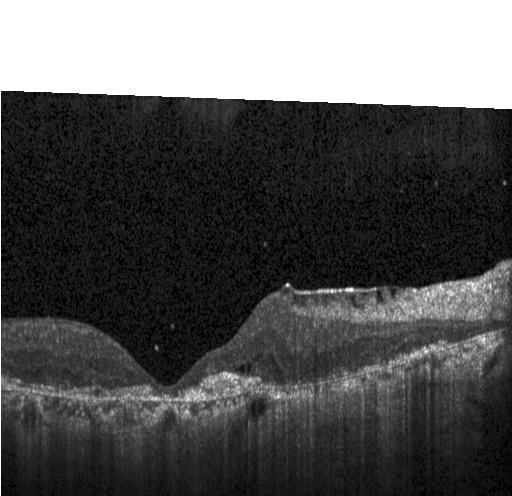 Diagnosis: choroidal neovascularization.